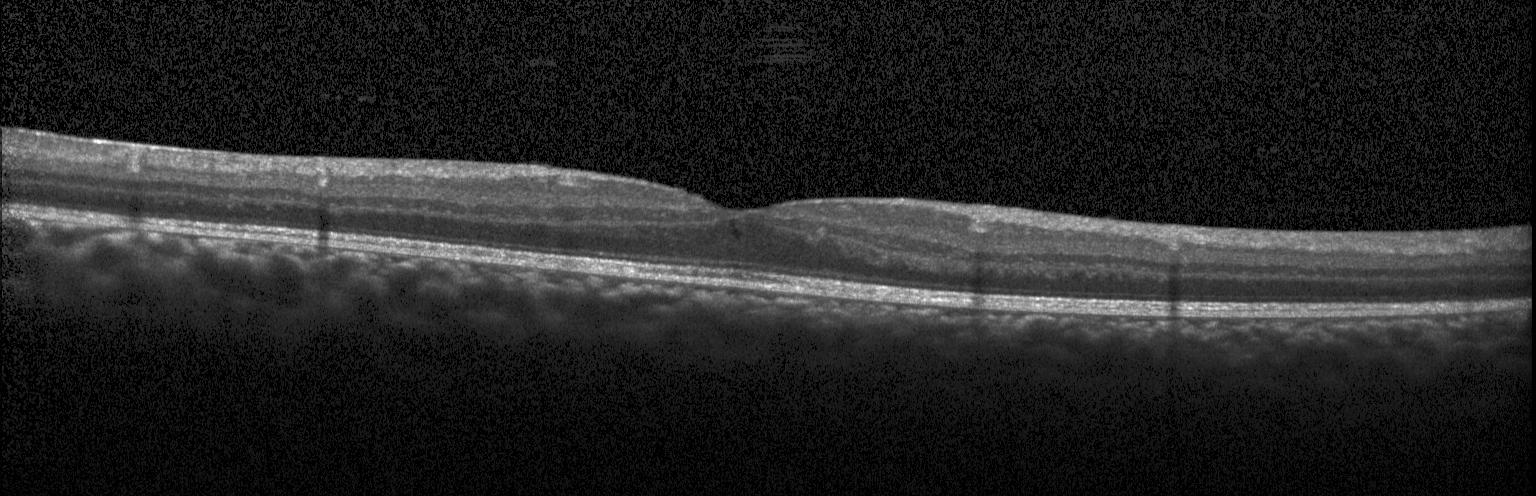 OCT line scan
Diagnosis: diabetic macular edema.